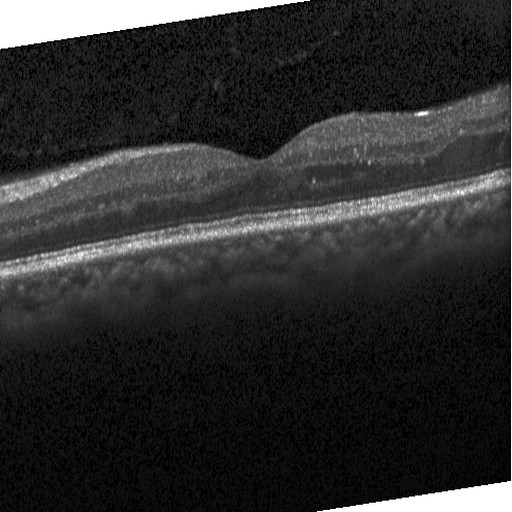

Spectral-domain OCT. Retinal OCT cross-section.
The scan shows diabetic macular edema (DME).